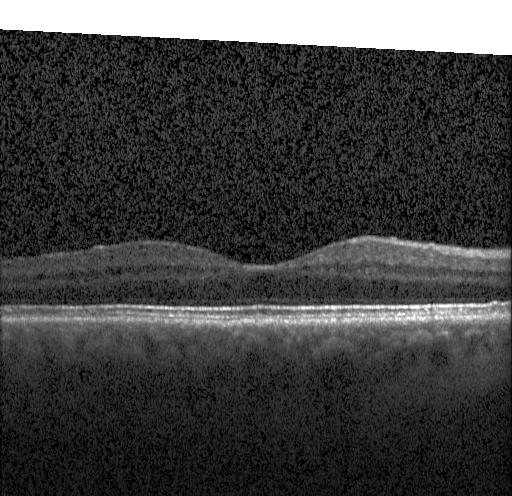
Macular scan. Instrument: Heidelberg Spectralis. Retinal OCT B-scan — Diagnosis: no evidence of choroidal neovascularization, diabetic macular edema, or drusen.